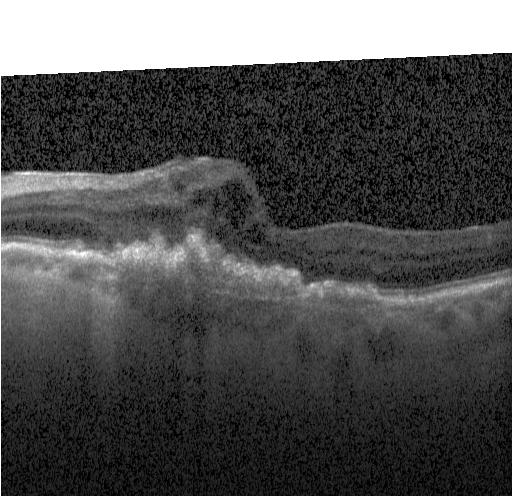
Heidelberg Spectralis · SD-OCT · OCT B-scan
This B-scan demonstrates a choroidal neovascular membrane.